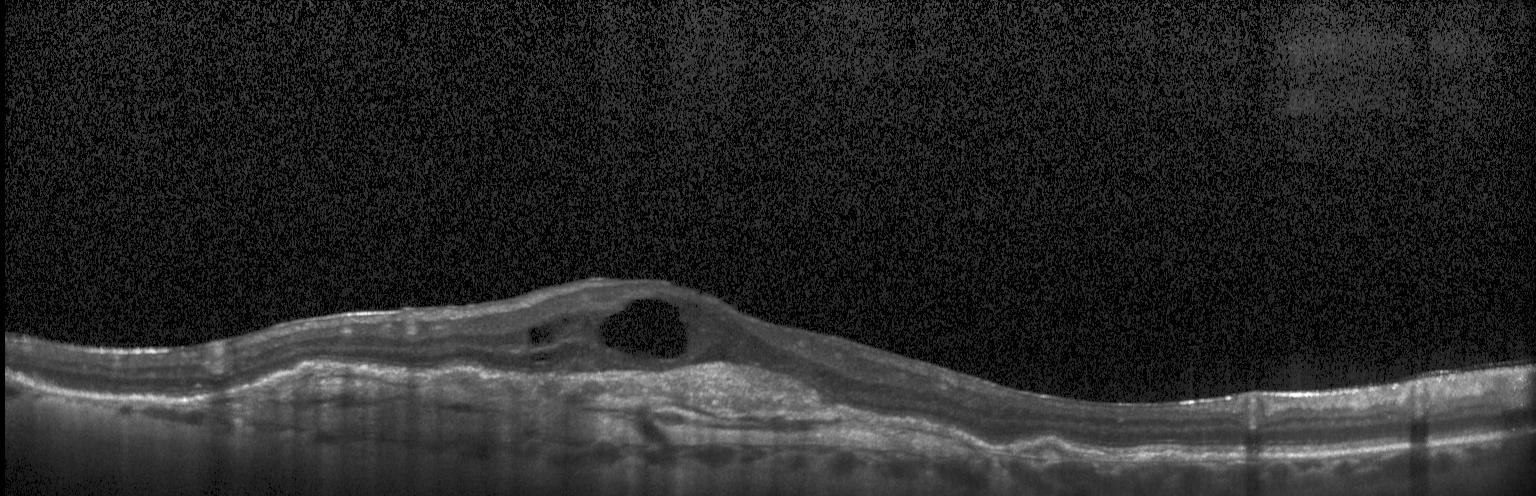 Instrument: Heidelberg Spectralis. OCT B-scan. SD-OCT. Horizontal scan through the fovea.
Finding: a choroidal neovascular membrane.